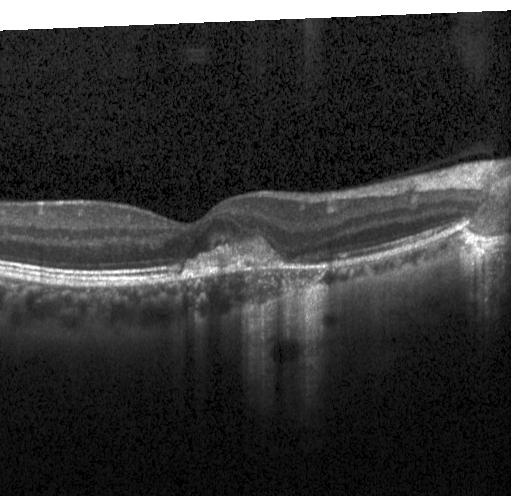
Heidelberg Spectralis OCT system, through the macula, SD-OCT, optical coherence tomography B-scan.
The scan shows a choroidal neovascular membrane.